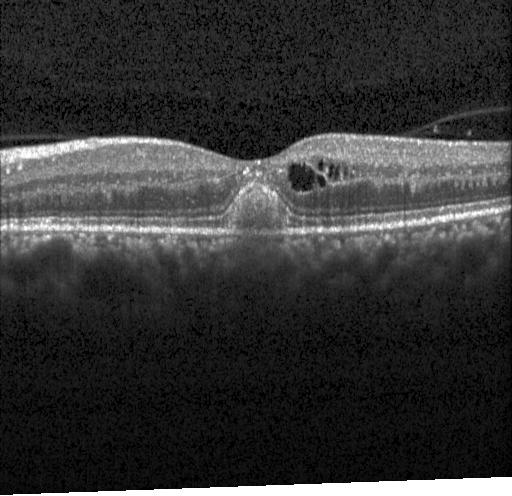 Instrument: Heidelberg Spectralis; OCT B-scan; through the macula. Diagnosis: choroidal neovascularization (CNV).